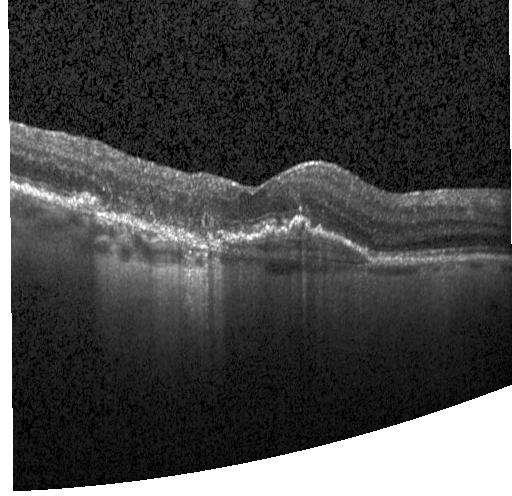
Diagnosis: a choroidal neovascular membrane.